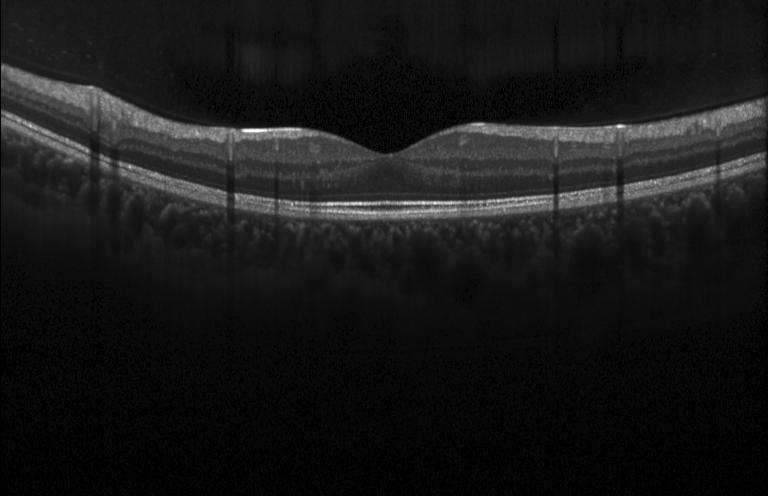 Spectral-domain OCT, retinal OCT cross-section, horizontal scan through the fovea, Heidelberg Spectralis OCT system
This B-scan demonstrates no evidence of CNV, DME, or drusen.